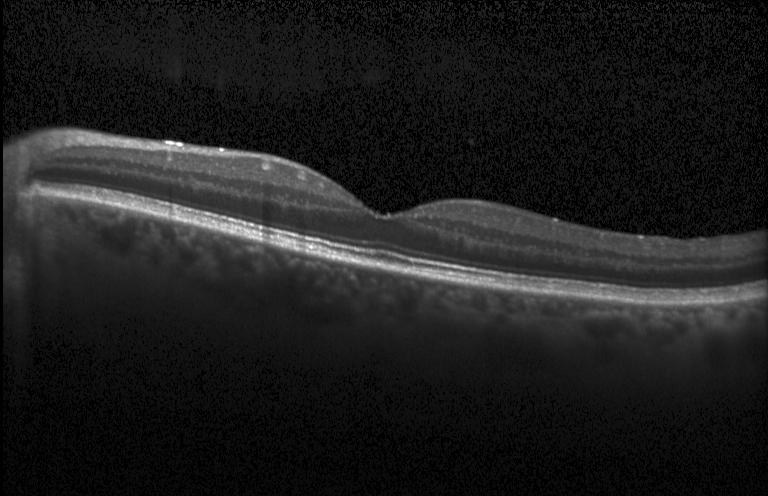
Heidelberg Spectralis, OCT B-scan.
No choroidal neovascularization, no diabetic macular edema, and no drusen.